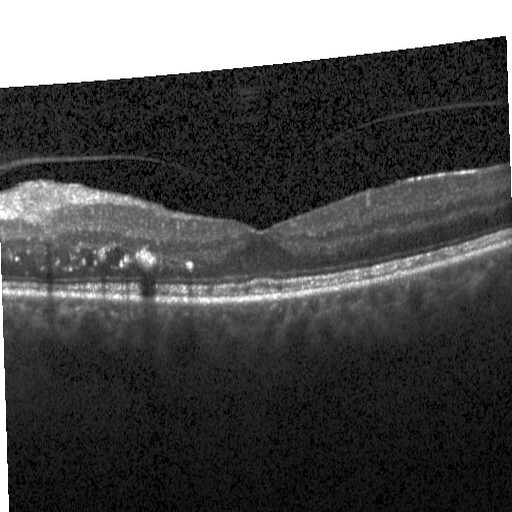
Impression: diabetic macular edema (DME).